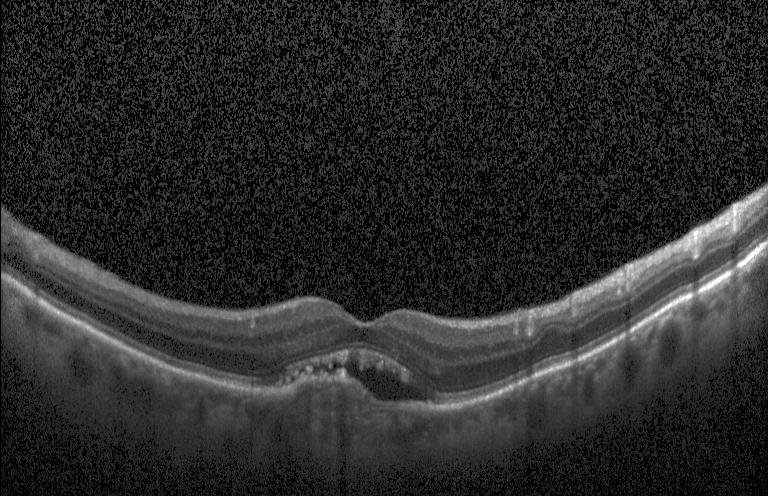

Heidelberg Spectralis, optical coherence tomography B-scan, macular scan, spectral-domain optical coherence tomography — A choroidal neovascular membrane.